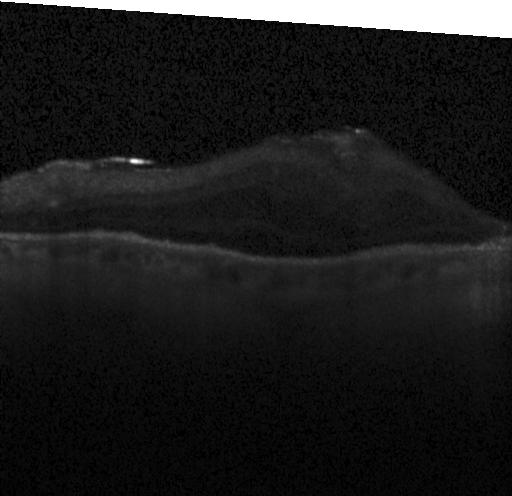

OCT B-scan, spectral-domain optical coherence tomography. CNV.